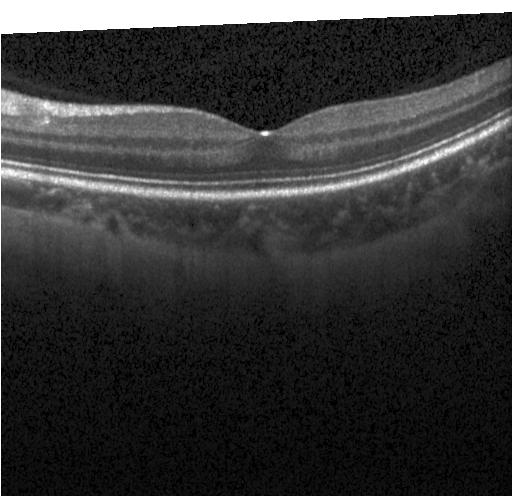
Heidelberg Spectralis; retinal OCT B-scan
Diagnosis: no evidence of choroidal neovascularization, diabetic macular edema, or drusen.